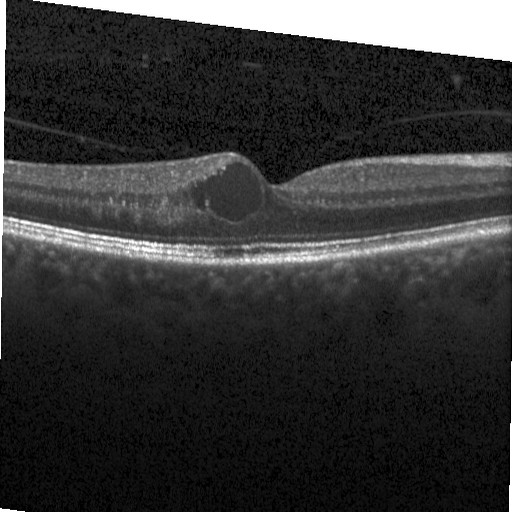
OCT B-scan showing diabetic macular edema (DME).